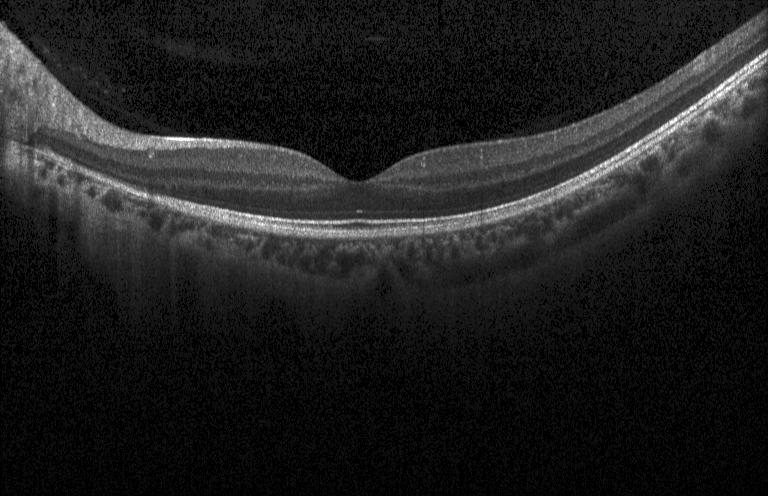
Optical coherence tomography scan — This B-scan demonstrates no choroidal neovascularization, diabetic macular edema, or drusen.